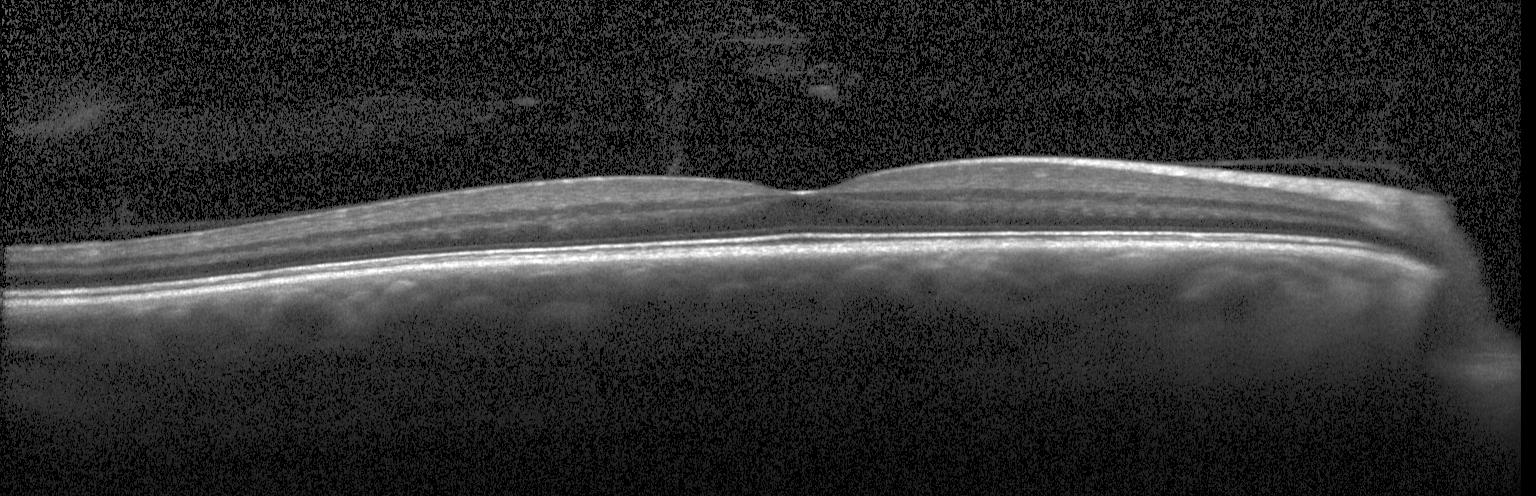
This B-scan demonstrates no CNV, no DME, and no drusen.